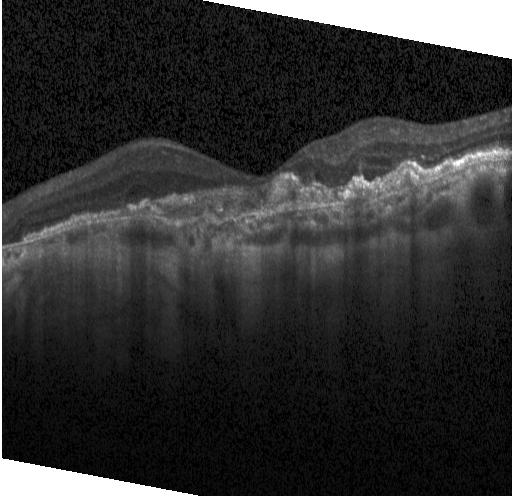 OCT B-scan showing a choroidal neovascular membrane.